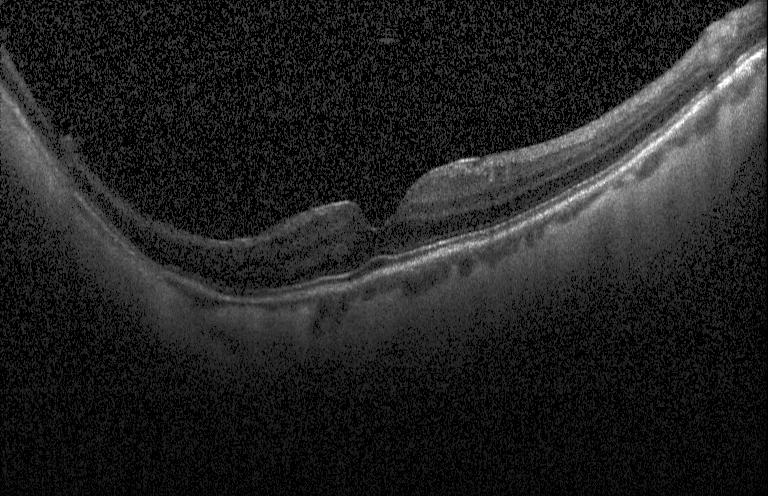

Retinal OCT cross-section. The scan shows no CNV, DME, or drusen.